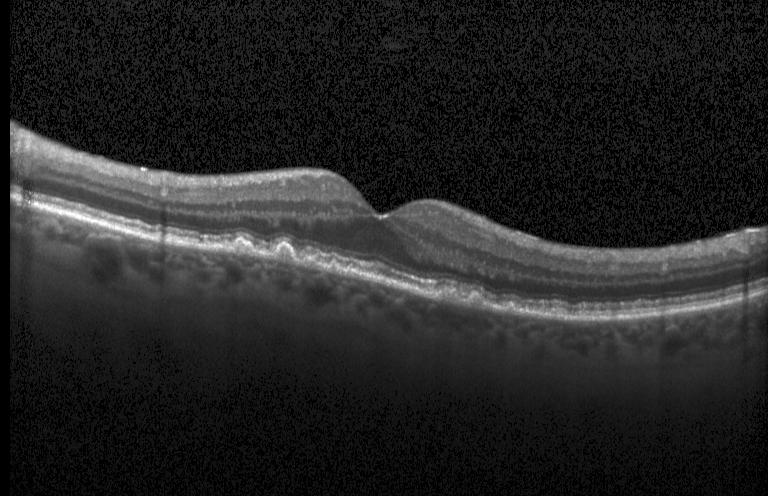

Dx: multiple drusen.